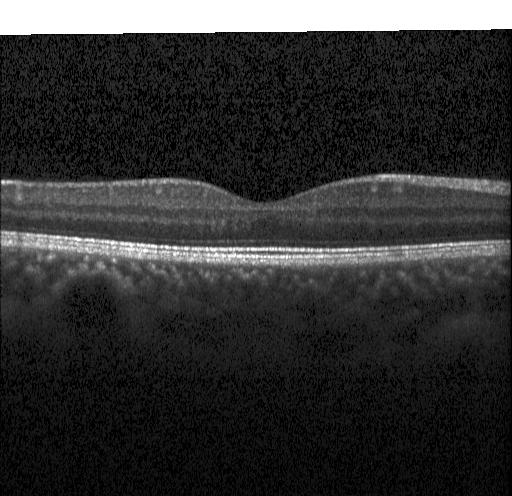
Optical coherence tomography scan
Impression: neither choroidal neovascularization, diabetic macular edema, nor drusen.